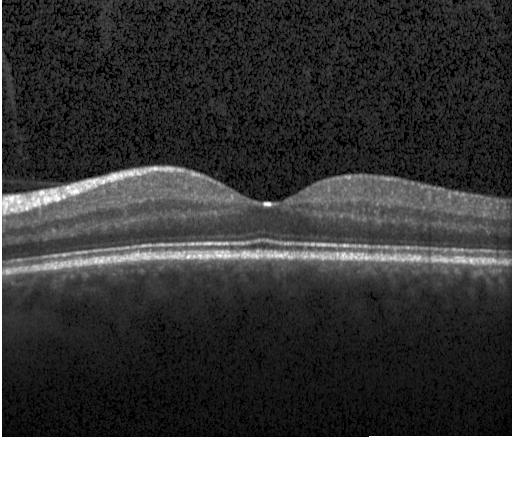 Retinal OCT cross-section.
Finding: no choroidal neovascularization, diabetic macular edema, or drusen.